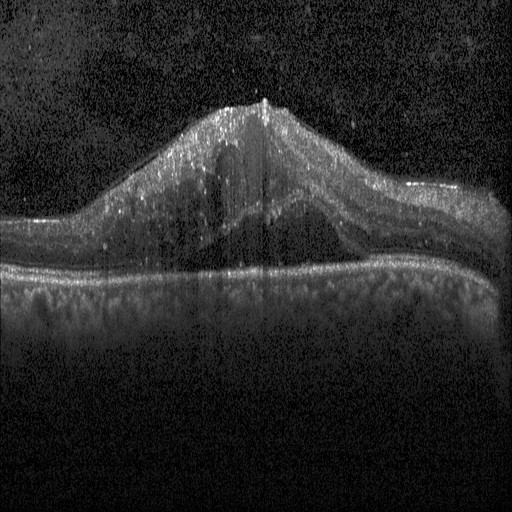 Impression: DME.